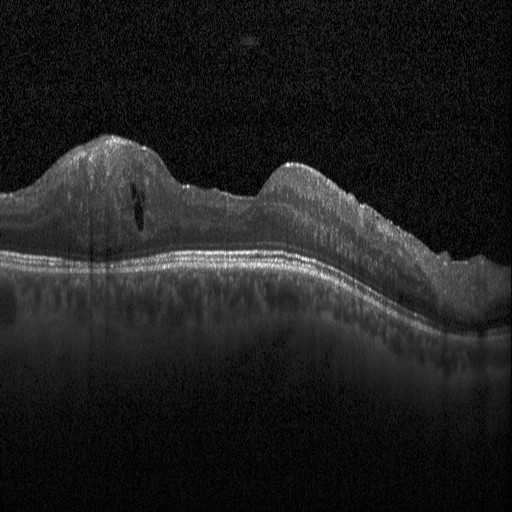
SD-OCT · acquired on a Heidelberg Spectralis · retinal OCT B-scan
Diagnosis: diabetic macular edema.